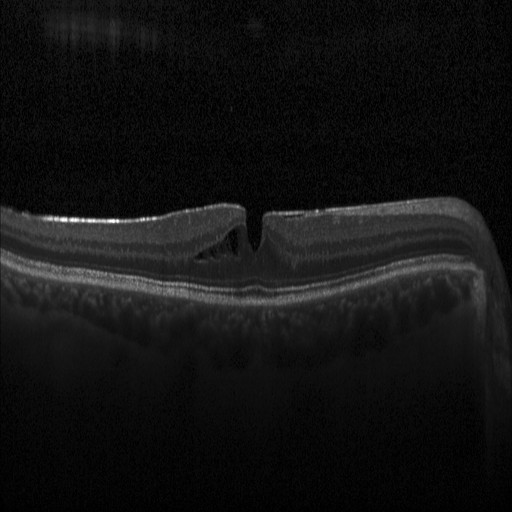 Retinal OCT cross-section. Spectral-domain OCT. Heidelberg Spectralis OCT system — Impression: diabetic macular edema.